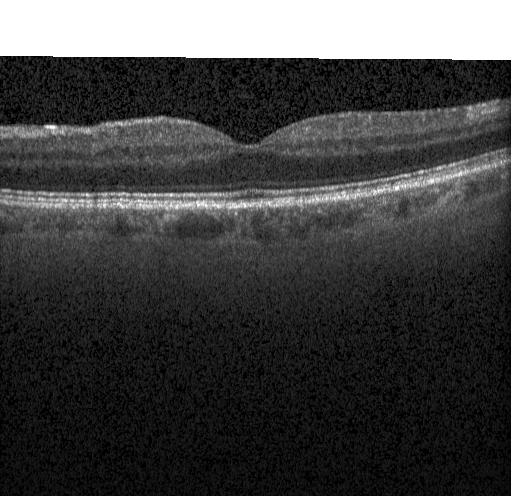
Optical coherence tomography scan — Neither CNV, DME, nor drusen.